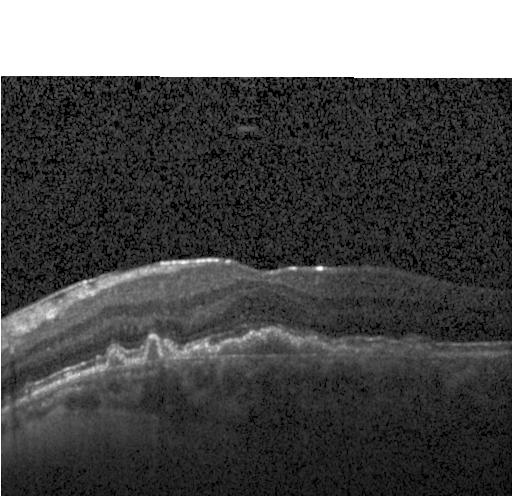

Heidelberg Spectralis, retinal OCT B-scan
CNV.